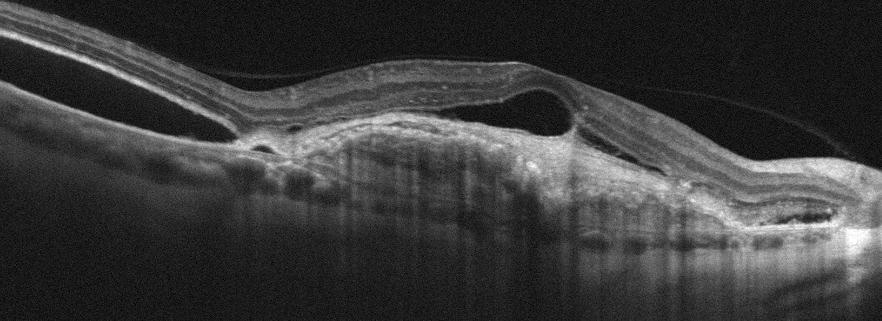

Macular scan · OCT line scan · Optovue Avanti RTVue XR. This B-scan demonstrates age-related macular degeneration.